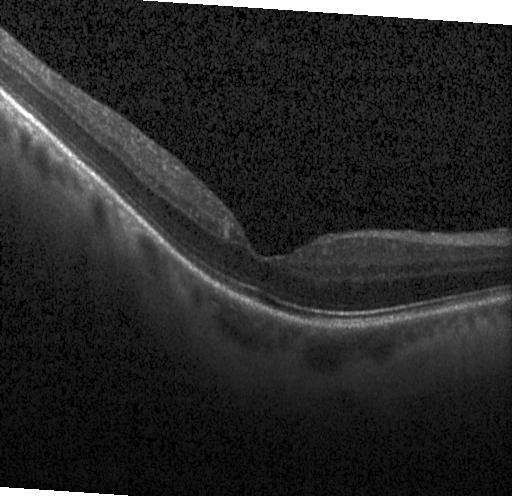 Retinal OCT B-scan, acquired on a Heidelberg Spectralis.
Dx: no CNV, no DME, and no drusen.